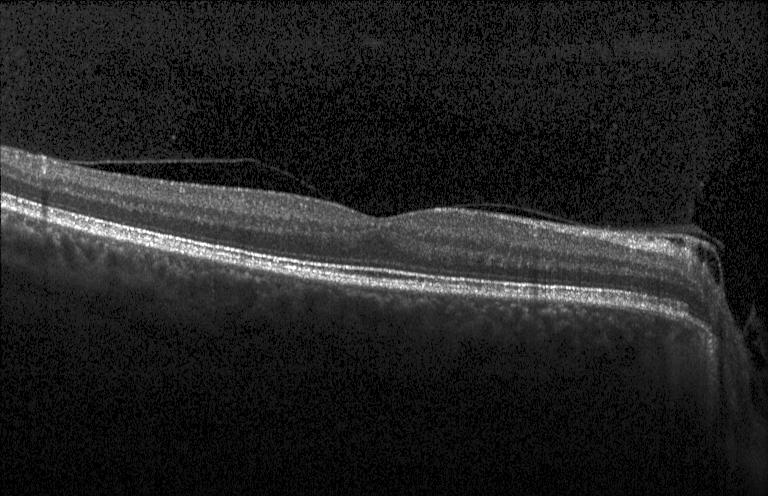 Acquired on a Heidelberg Spectralis; spectral-domain OCT; optical coherence tomography B-scan; through the macula. Impression: no evidence of choroidal neovascularization, diabetic macular edema, or drusen.